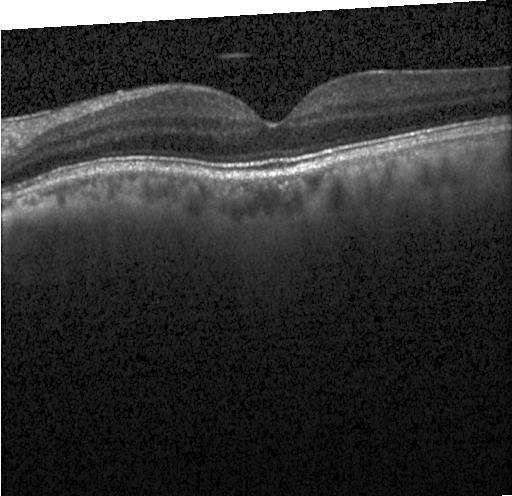

Impression: no evidence of choroidal neovascularization, diabetic macular edema, or drusen.